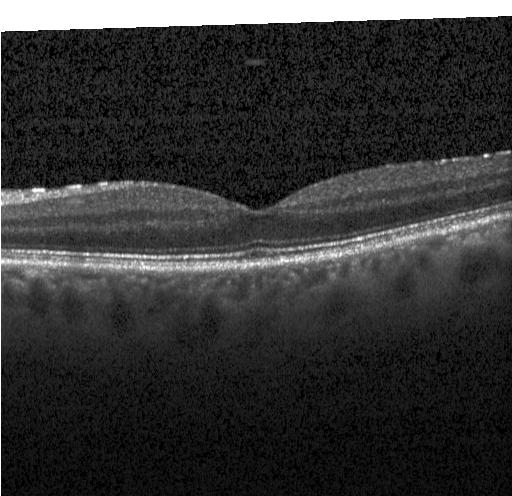 Optical coherence tomography scan
Finding: no evidence of CNV, DME, or drusen.